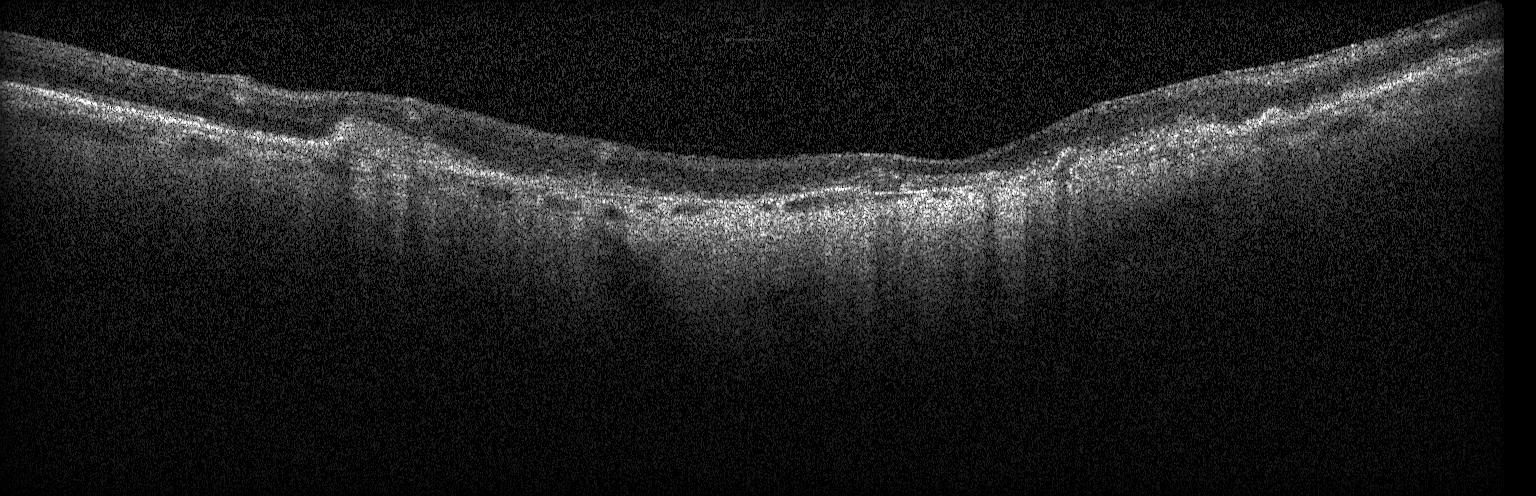 Spectral-domain optical coherence tomography; OCT line scan; horizontal scan through the fovea
Macular OCT: choroidal neovascularization.